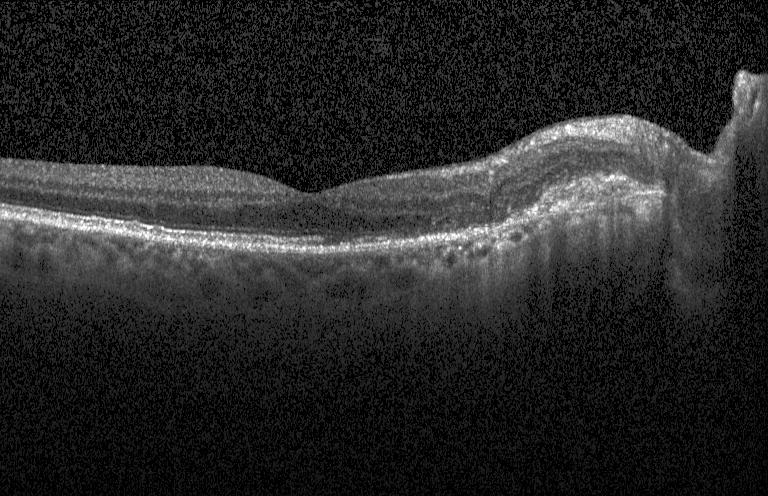
Spectral-domain optical coherence tomography · retinal OCT B-scan · horizontal scan through the fovea · Heidelberg Spectralis OCT system.
Diagnosis: choroidal neovascularization.